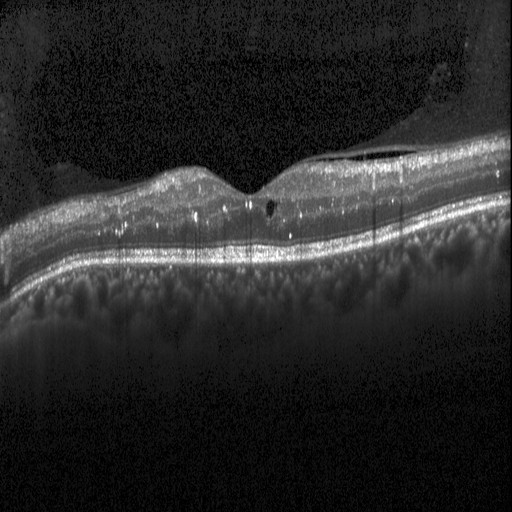
Macular scan · OCT line scan. Diabetic macular edema (DME).